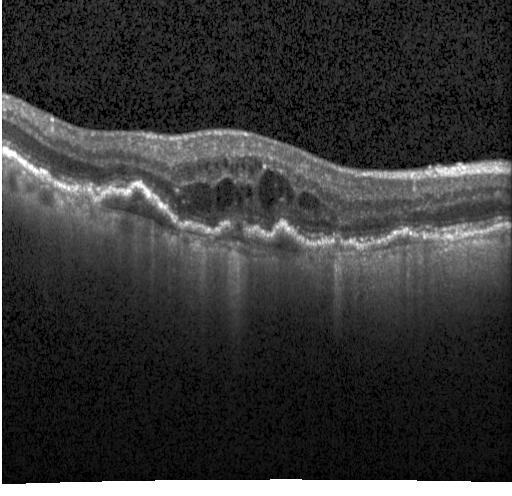
Finding: a choroidal neovascular membrane.